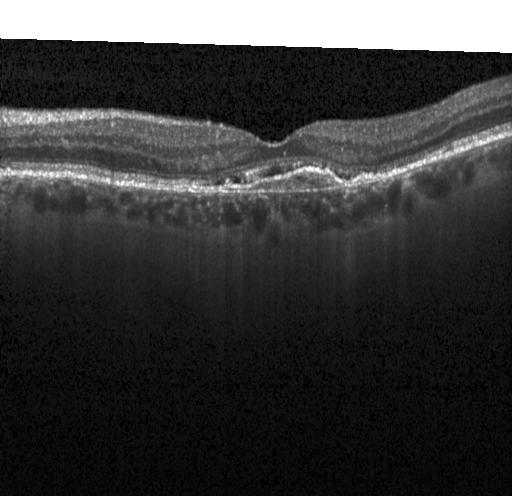 Heidelberg Spectralis. Retinal OCT B-scan — The scan shows choroidal neovascularization.